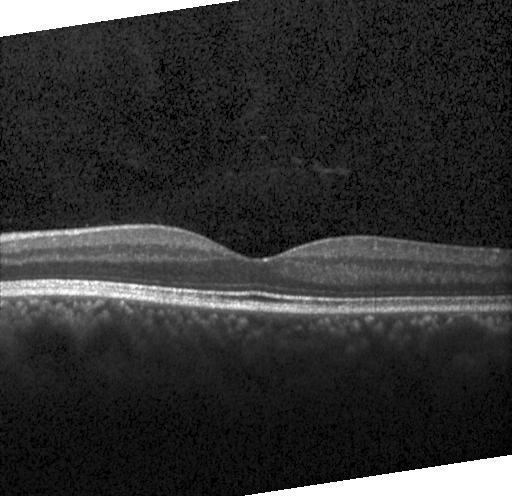 Diagnosis: no evidence of choroidal neovascularization, diabetic macular edema, or drusen.